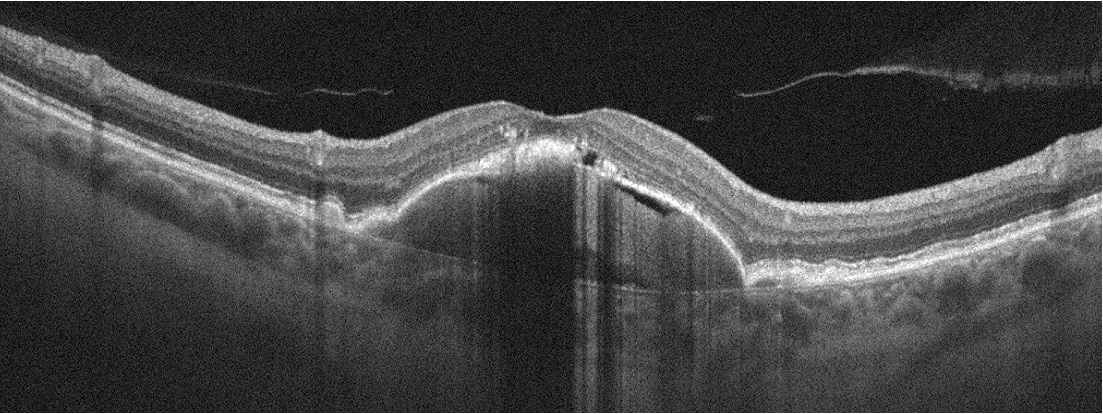 Dx: age-related macular degeneration.